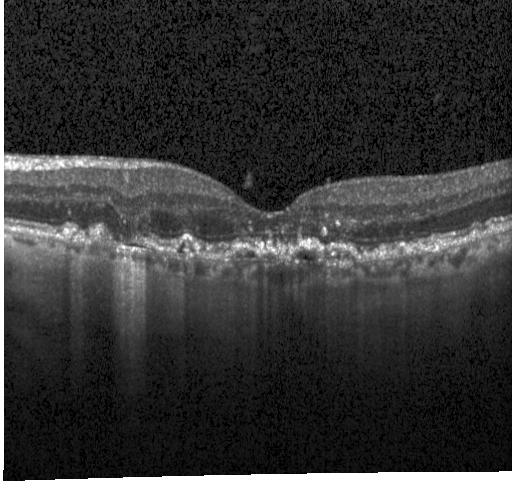 Optical coherence tomography scan. Assessment: a choroidal neovascular membrane.